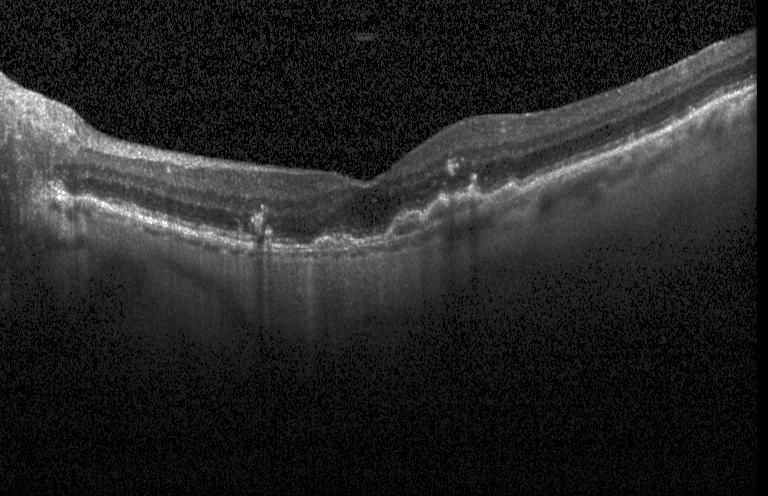 Impression: a choroidal neovascular membrane.